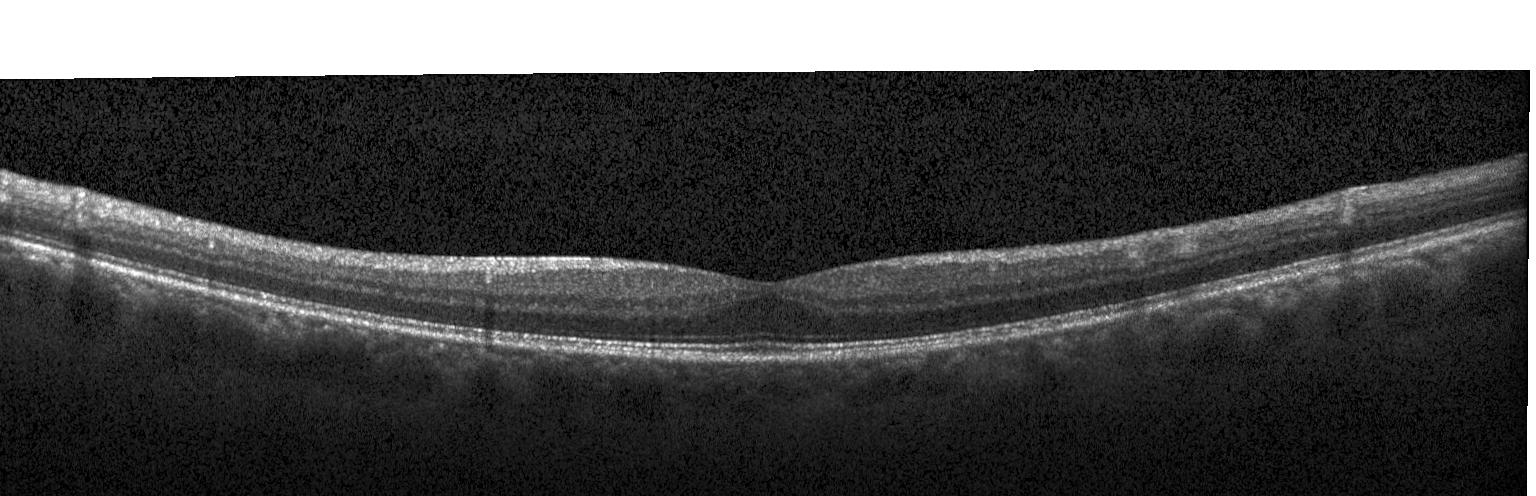

Retinal OCT cross-section showing no CNV, DME, or drusen.